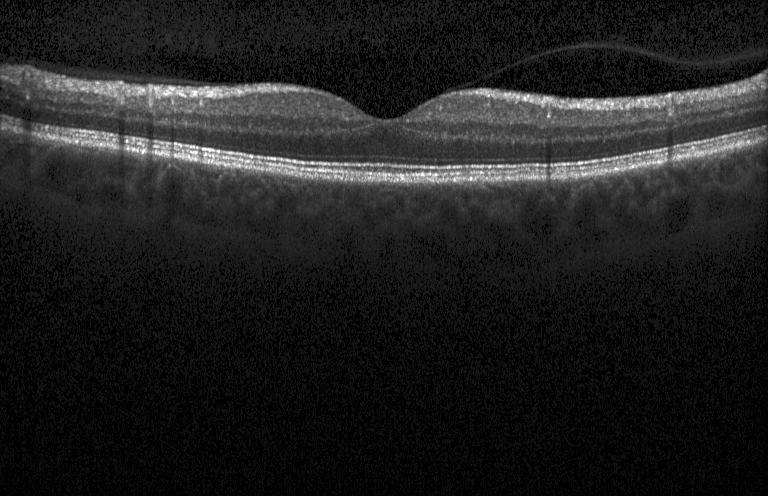 Optical coherence tomography B-scan.
Diagnosis: neither choroidal neovascularization, diabetic macular edema, nor drusen.